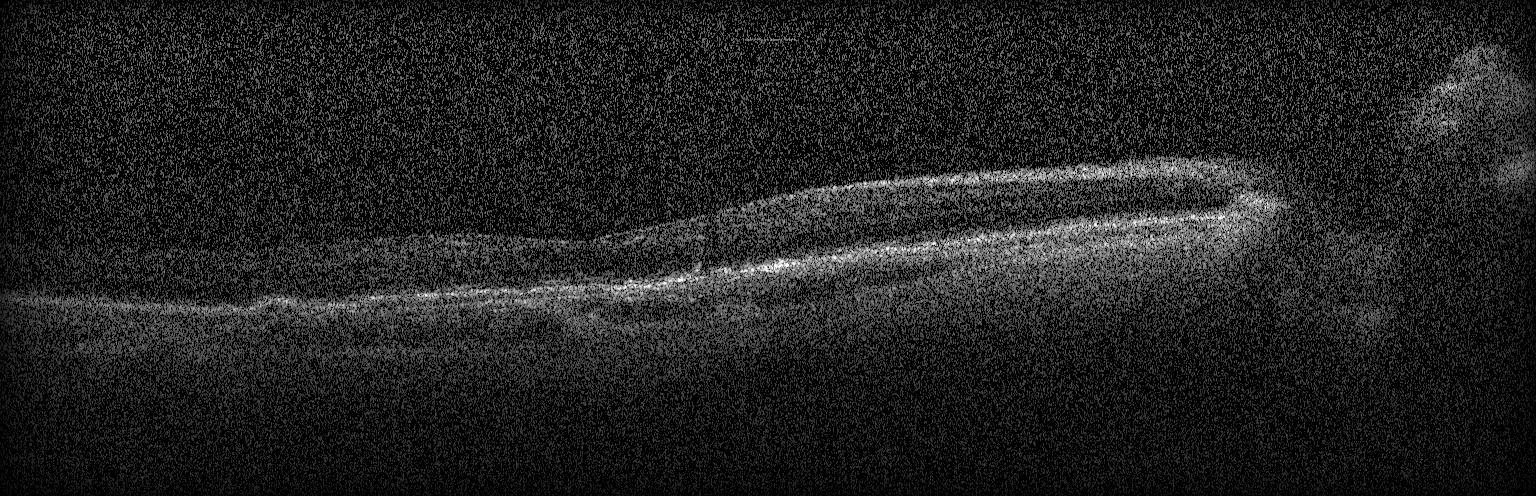

Impression: choroidal neovascularization.